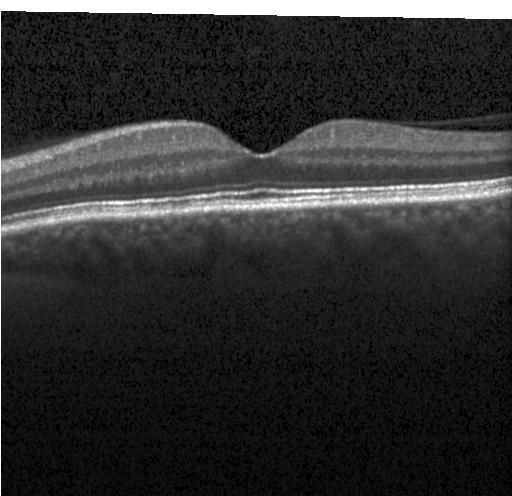
SD-OCT · horizontal scan through the fovea · OCT B-scan · Heidelberg Spectralis OCT system.
No evidence of choroidal neovascularization, diabetic macular edema, or drusen.